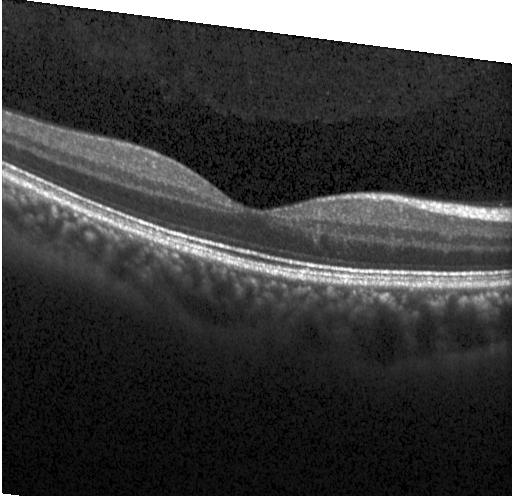
Retinal OCT cross-section.
This B-scan demonstrates neither CNV, DME, nor drusen.